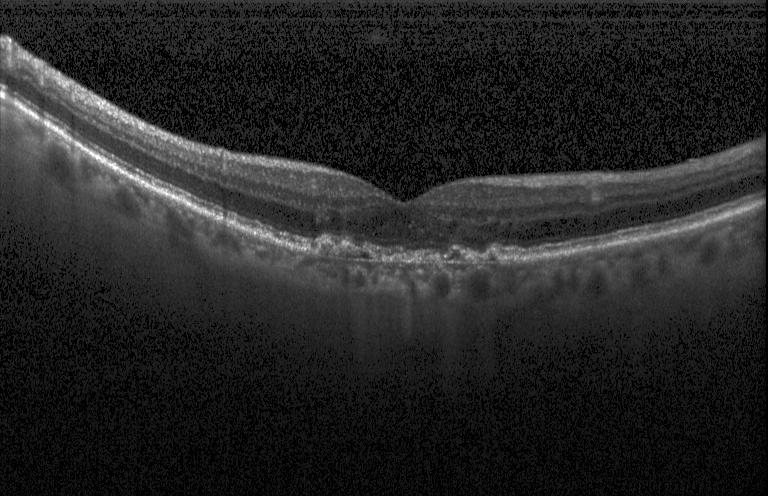 Spectral-domain OCT; OCT line scan; centered on the fovea; Heidelberg Spectralis OCT system
Finding: drusen.